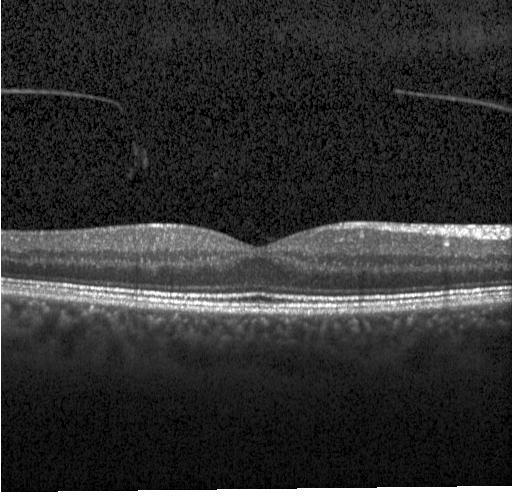
Optical coherence tomography scan.
Impression: no choroidal neovascularization, diabetic macular edema, or drusen.